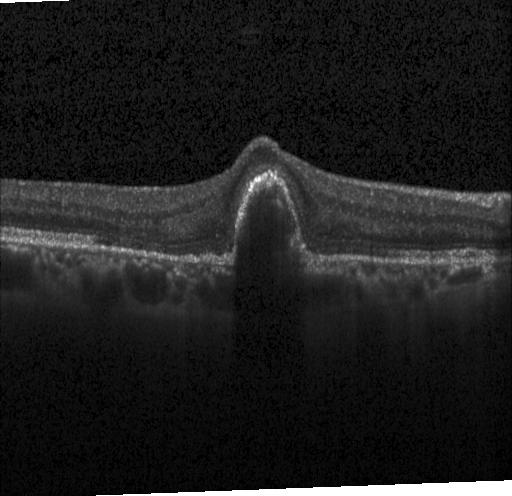 Retinal OCT cross-section showing a choroidal neovascular membrane.